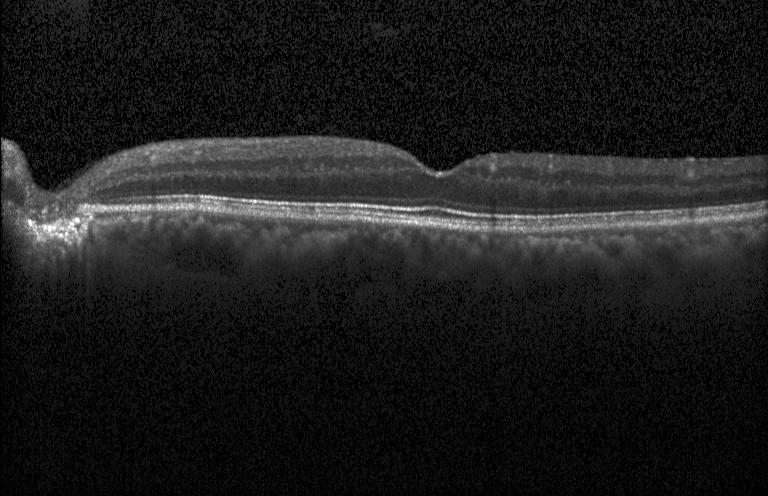
Macular OCT: no choroidal neovascularization, diabetic macular edema, or drusen.